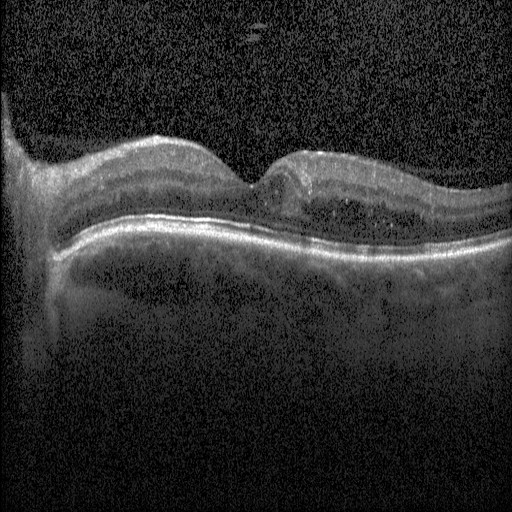
Optical coherence tomography B-scan. Centered on the fovea. Instrument: Heidelberg Spectralis. OCT finding: diabetic macular edema.